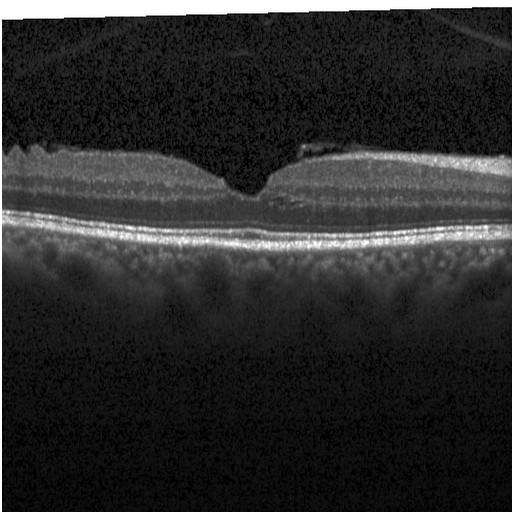 Finding: diabetic macular edema.